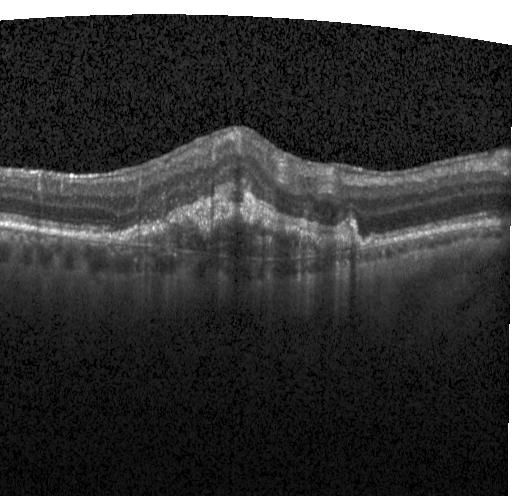

Diagnosis: a choroidal neovascular membrane.